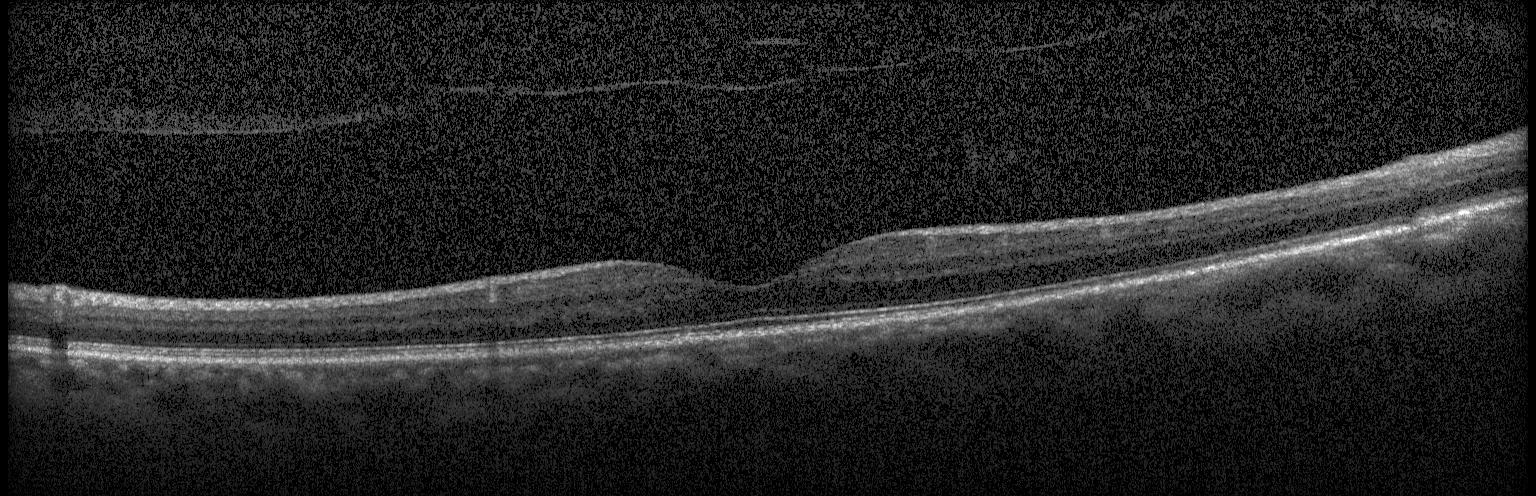 Retinal OCT B-scan — OCT finding: neither CNV, DME, nor drusen.